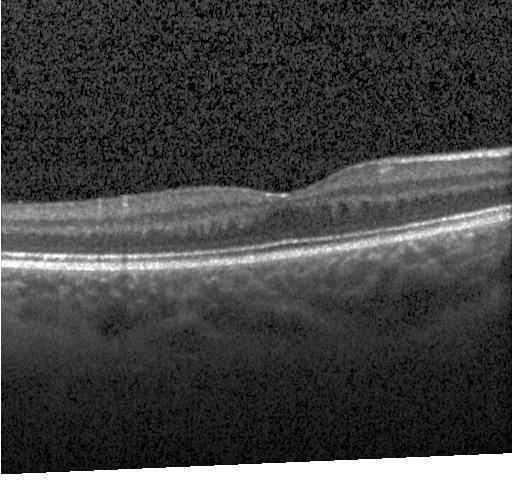 Retinal OCT cross-section; centered on the fovea; acquired on a Heidelberg Spectralis
The scan shows no evidence of choroidal neovascularization, diabetic macular edema, or drusen.